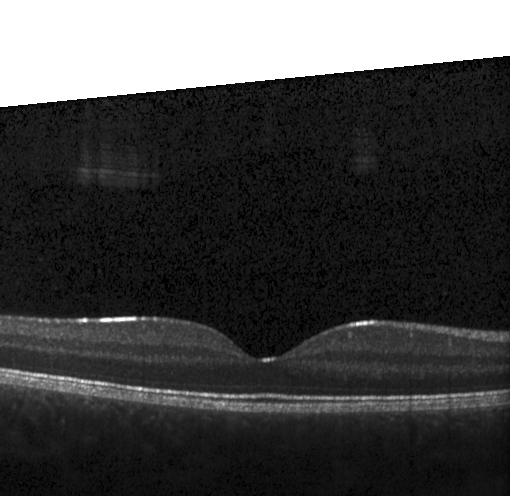

Optical coherence tomography scan · Heidelberg Spectralis OCT system · macular scan.
Diagnosis: no CNV, no DME, and no drusen.